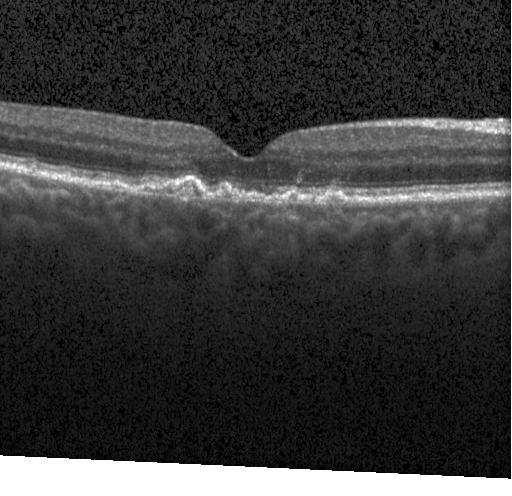
OCT finding: choroidal neovascularization (CNV).